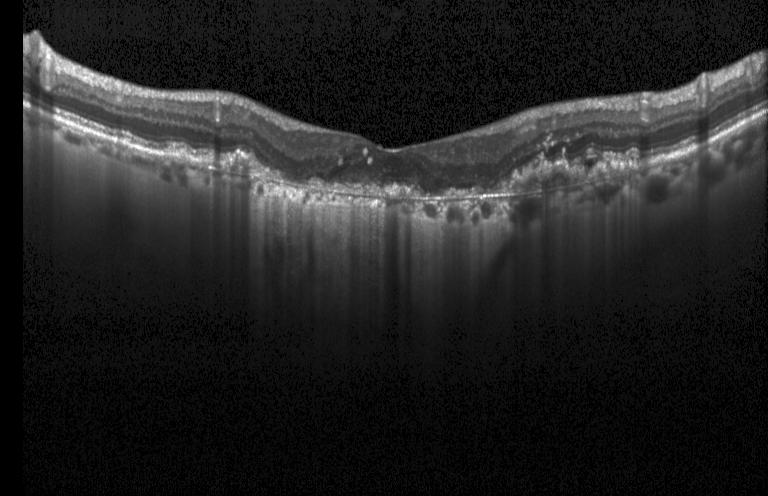
Finding: a choroidal neovascular membrane.